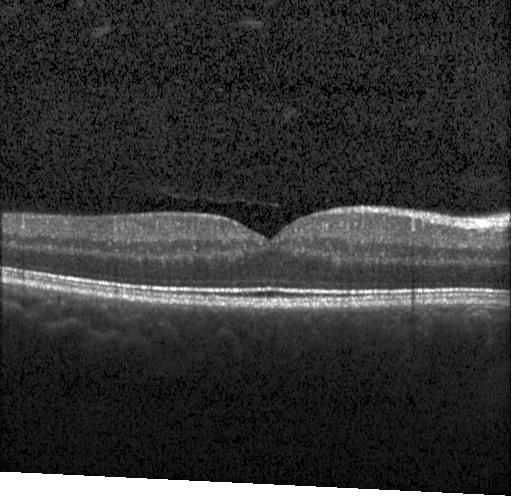 Retinal OCT cross-section. Finding: no choroidal neovascularization, no diabetic macular edema, and no drusen.